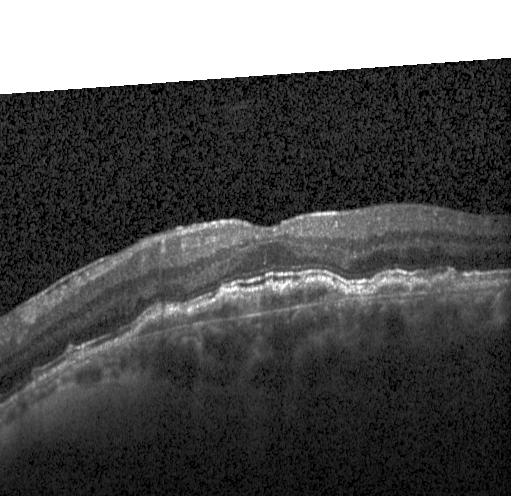 OCT B-scan showing a choroidal neovascular membrane.